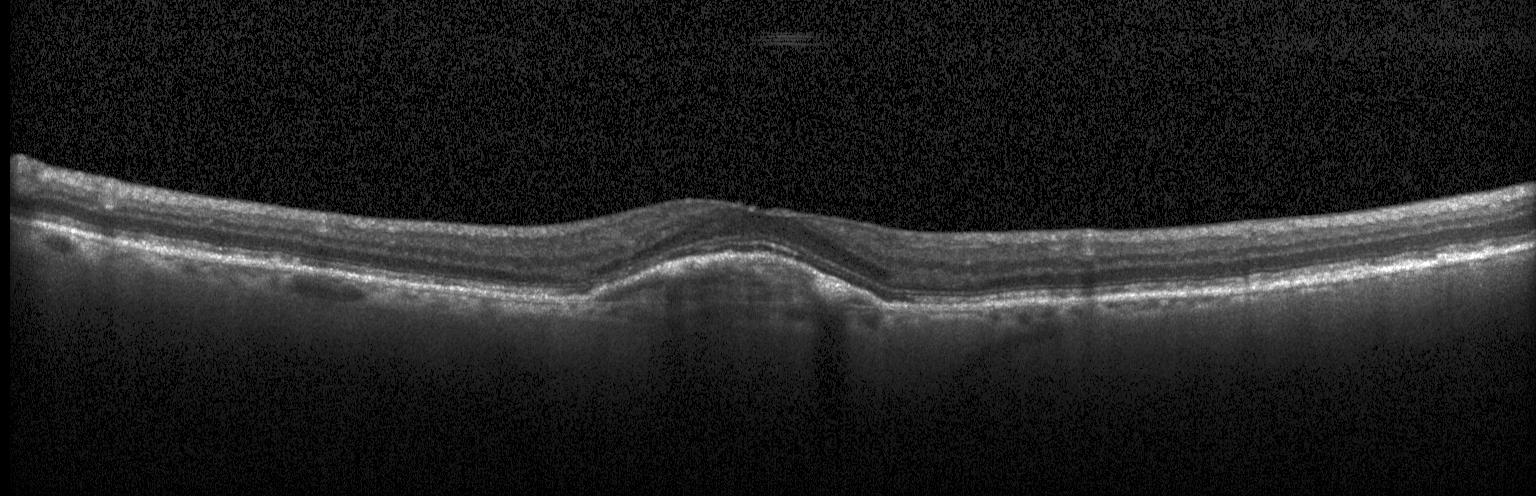 Centered on the fovea; OCT B-scan
Finding: a choroidal neovascular membrane.